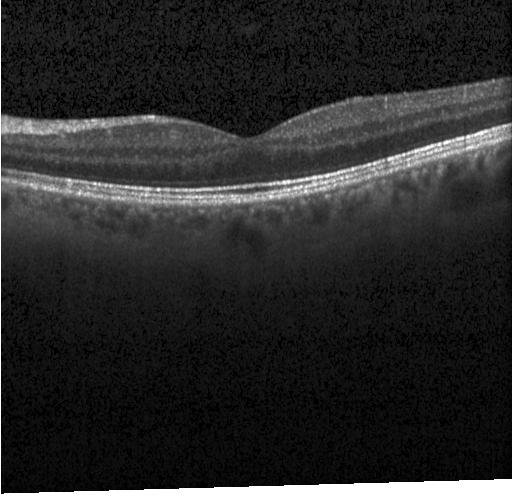 Finding: no choroidal neovascularization, diabetic macular edema, or drusen.